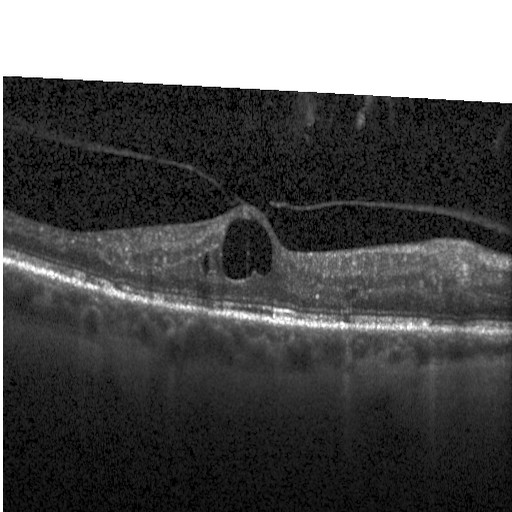
Acquired on a Heidelberg Spectralis; horizontal scan through the fovea; spectral-domain OCT; optical coherence tomography B-scan
OCT finding: diabetic macular edema (DME).